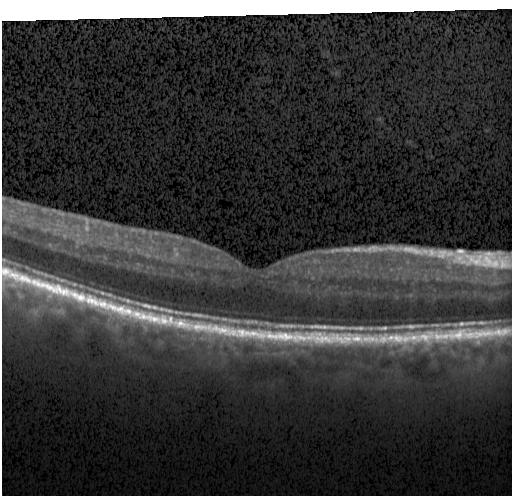 Retinal OCT cross-section
No evidence of choroidal neovascularization, diabetic macular edema, or drusen.